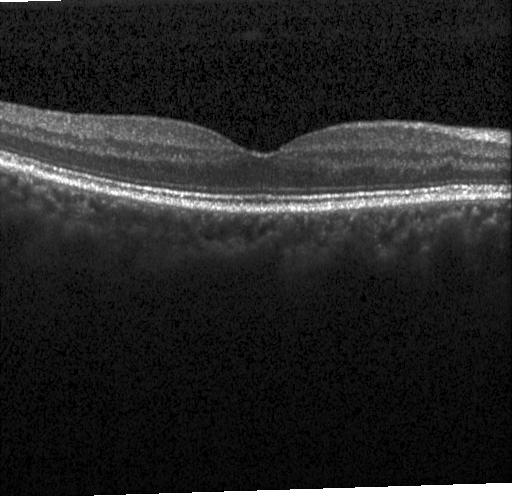

OCT B-scan
This B-scan demonstrates no CNV, DME, or drusen.